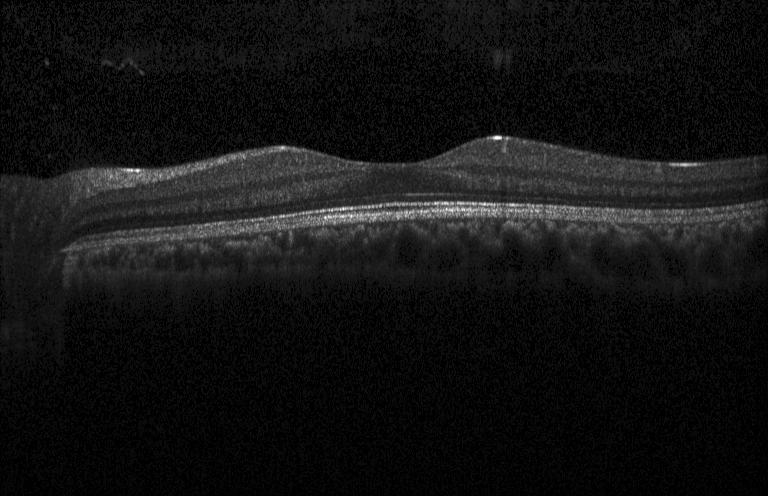
Heidelberg Spectralis · retinal OCT cross-section · SD-OCT · horizontal scan through the fovea
Finding: no evidence of choroidal neovascularization, diabetic macular edema, or drusen.